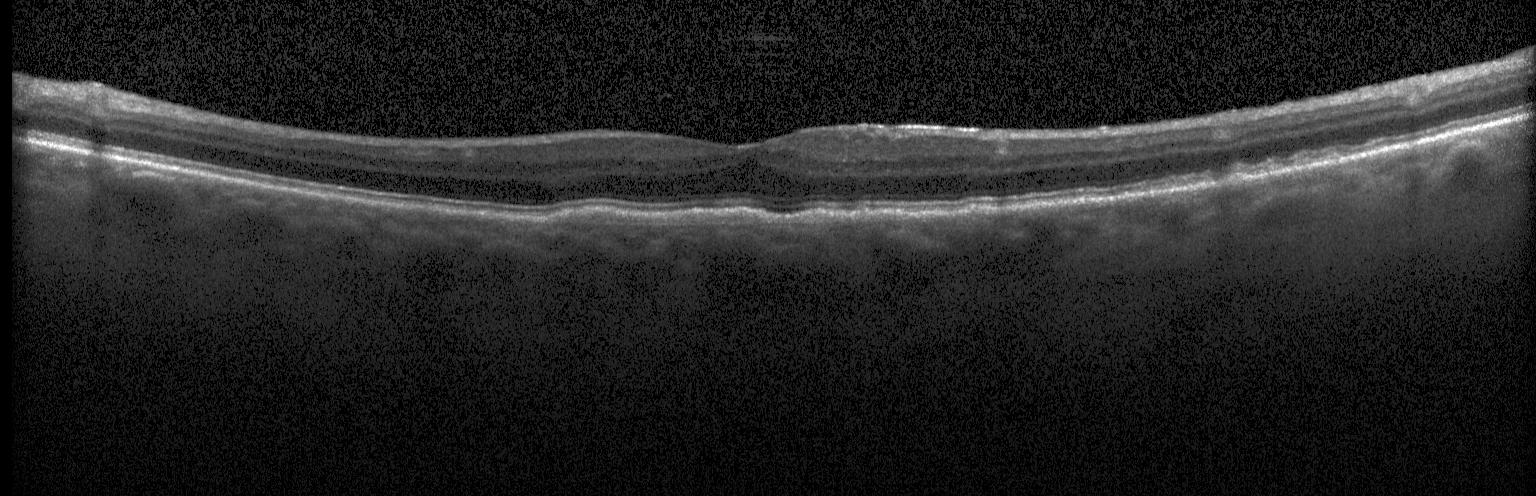 Dx: a choroidal neovascular membrane.